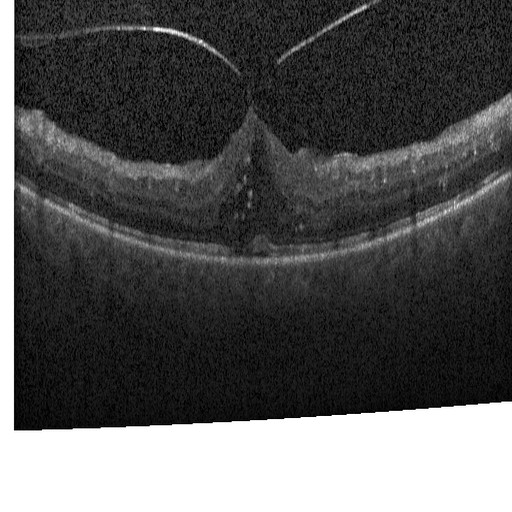
Horizontal scan through the fovea. OCT B-scan. Spectral-domain OCT. Heidelberg Spectralis OCT system.
Impression: diabetic macular edema (DME).